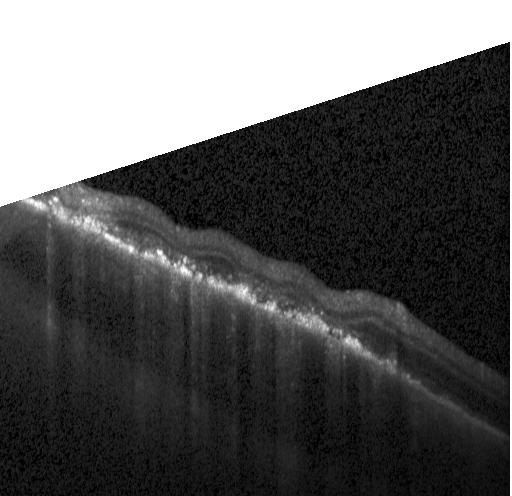 OCT B-scan. Spectral-domain optical coherence tomography — Diagnosis: a choroidal neovascular membrane.